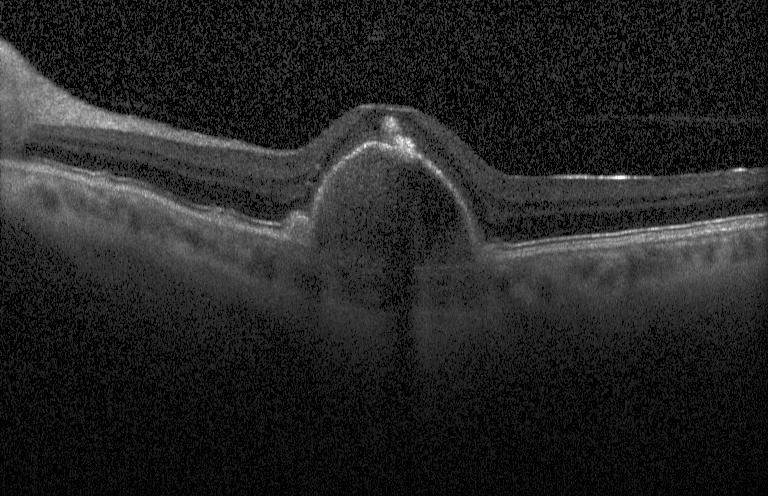 Macular OCT demonstrating choroidal neovascularization (CNV).